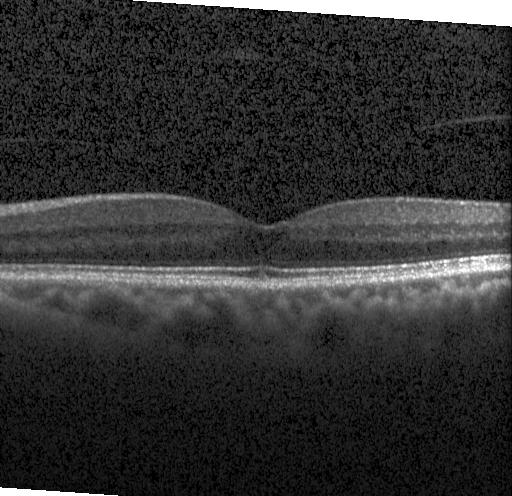 Macular OCT: no choroidal neovascularization, diabetic macular edema, or drusen.